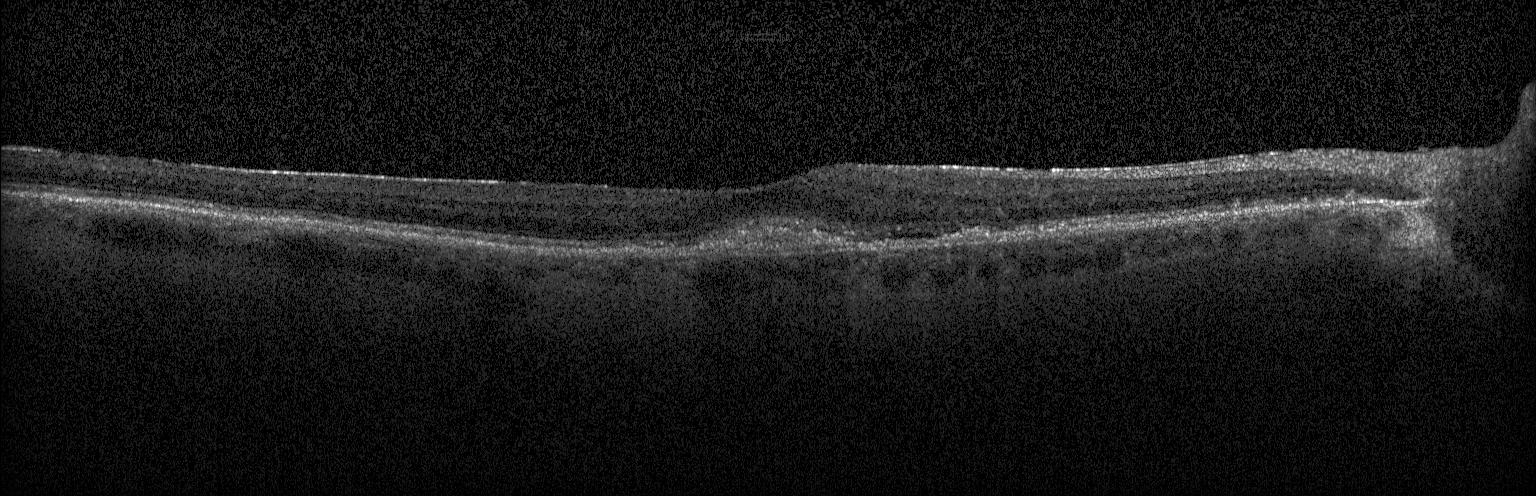
Spectral-domain optical coherence tomography, retinal OCT B-scan, centered on the fovea — OCT finding: a choroidal neovascular membrane.